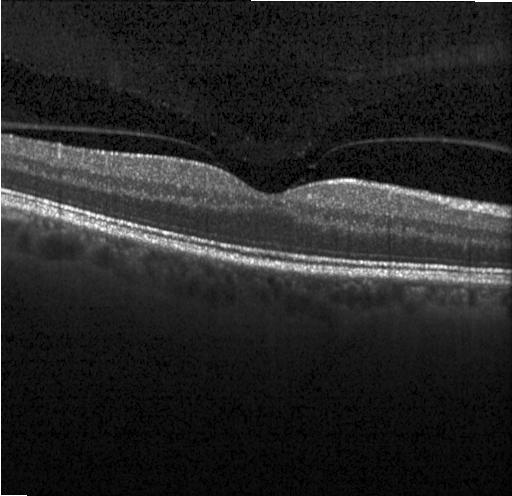
SD-OCT, Heidelberg Spectralis, fovea-centered, OCT B-scan
Diagnosis: no evidence of choroidal neovascularization, diabetic macular edema, or drusen.